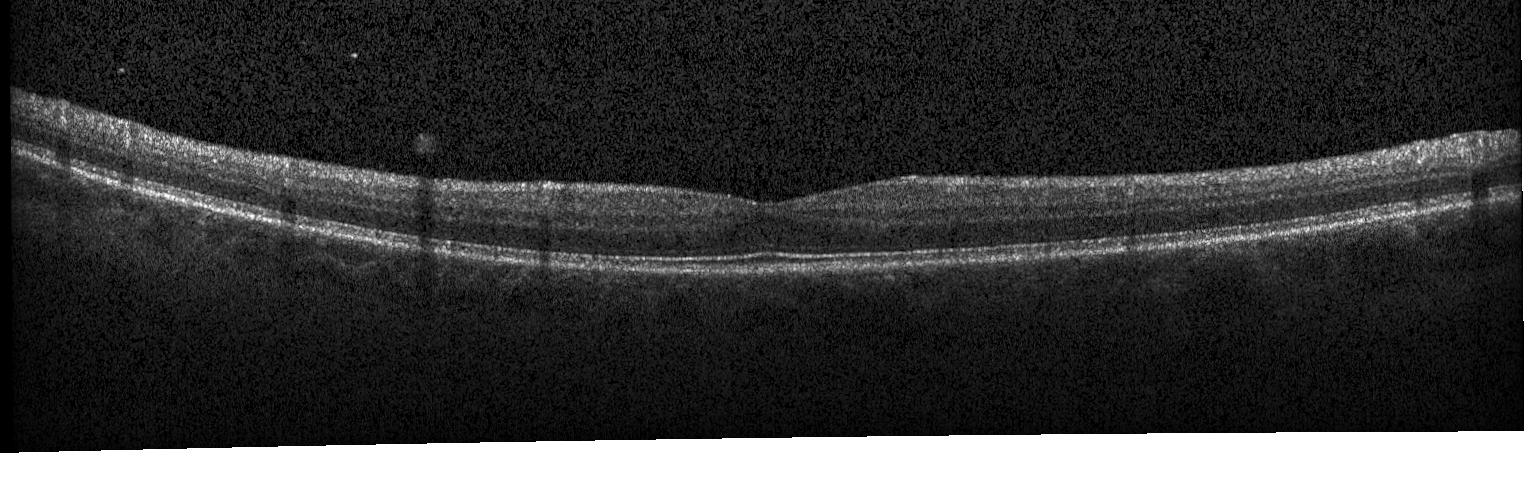
Impression: no evidence of choroidal neovascularization, diabetic macular edema, or drusen.